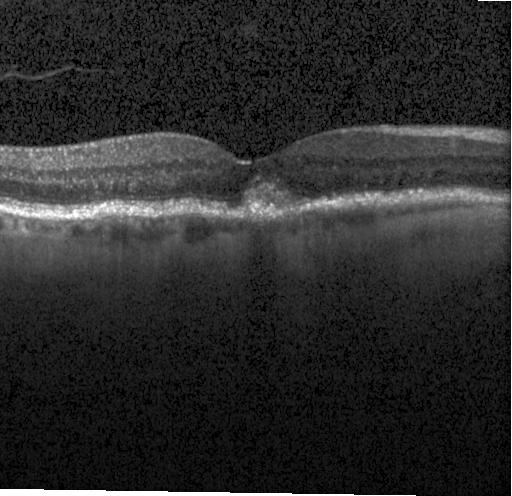 Macular OCT: multiple drusen.